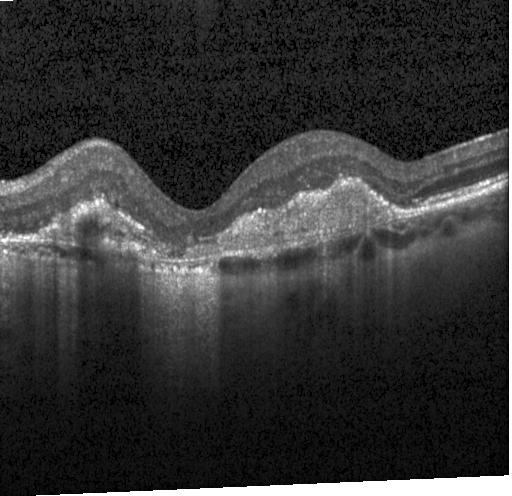
Spectral-domain optical coherence tomography. Optical coherence tomography B-scan. Through the macula — Dx: a choroidal neovascular membrane.